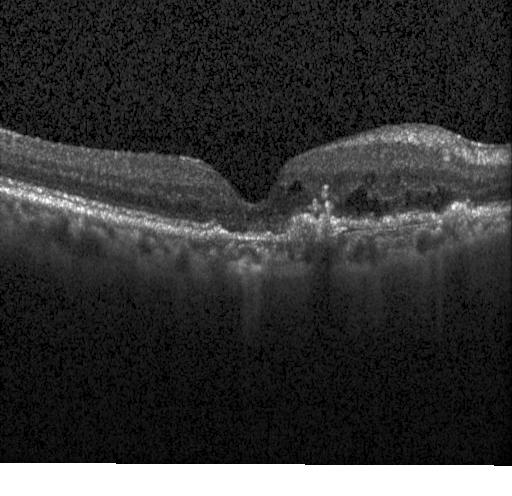
OCT B-scan · fovea-centered. Finding: choroidal neovascularization (CNV).